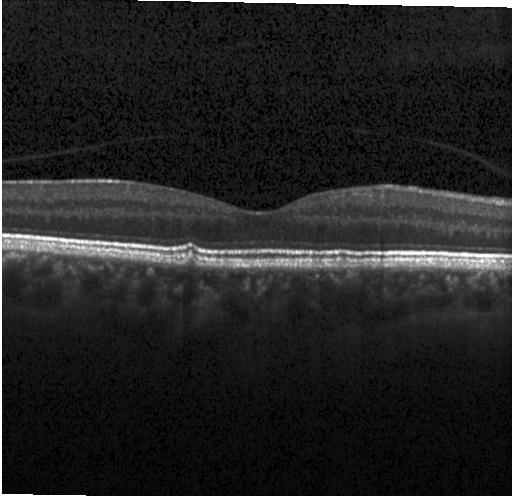 OCT line scan. Heidelberg Spectralis. Spectral-domain optical coherence tomography. Finding: multiple drusen.